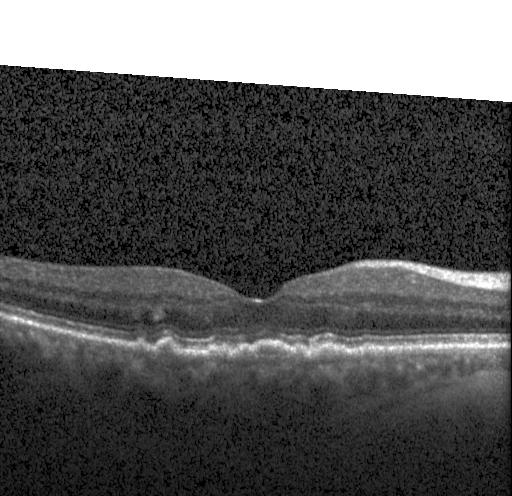 Optical coherence tomography B-scan, SD-OCT.
Macular OCT: sub-RPE drusenoid deposits.